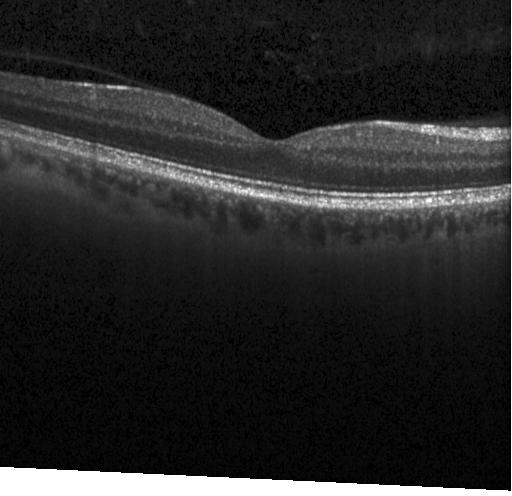 Spectral-domain OCT · macular scan · acquired on a Heidelberg Spectralis · optical coherence tomography B-scan. This B-scan demonstrates no choroidal neovascularization, diabetic macular edema, or drusen.